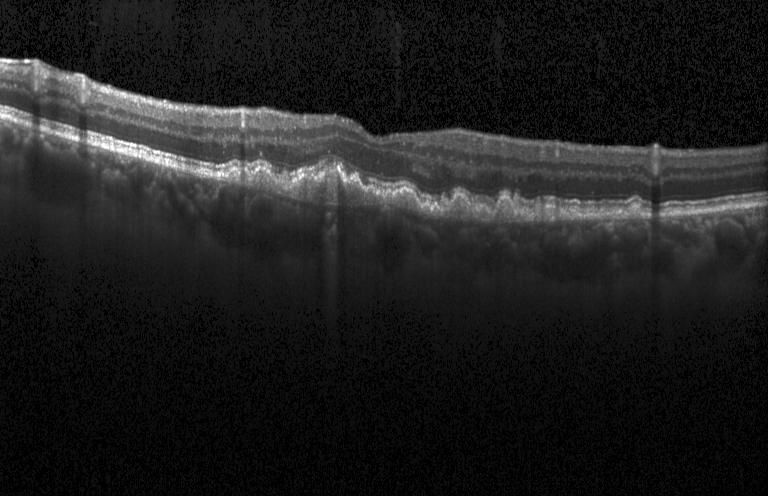 Horizontal scan through the fovea, retinal OCT cross-section, instrument: Heidelberg Spectralis
Finding: a choroidal neovascular membrane.